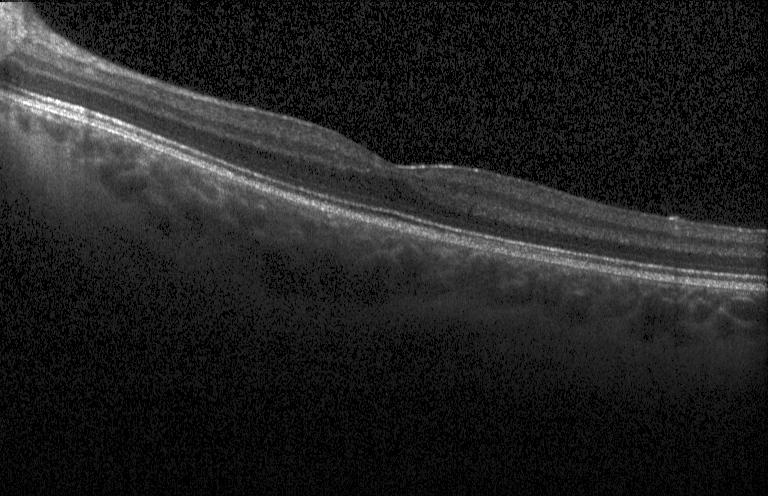

Optical coherence tomography scan
Impression: no choroidal neovascularization, diabetic macular edema, or drusen.